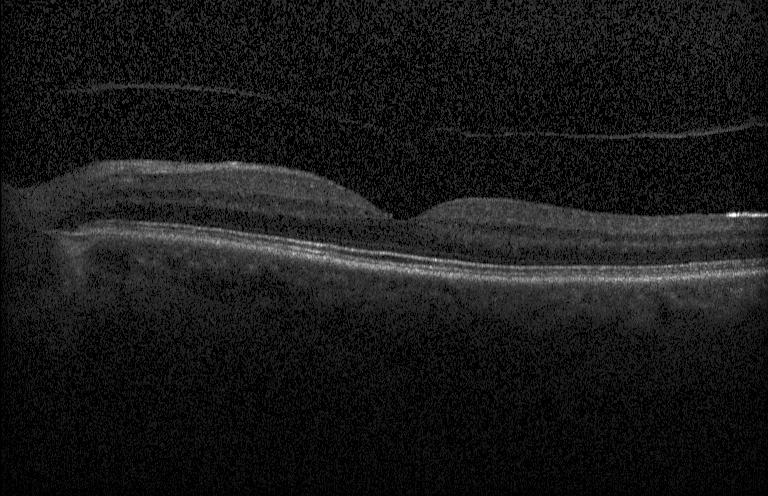 Spectral-domain optical coherence tomography. OCT line scan. Horizontal scan through the fovea.
The scan shows no evidence of choroidal neovascularization, diabetic macular edema, or drusen.